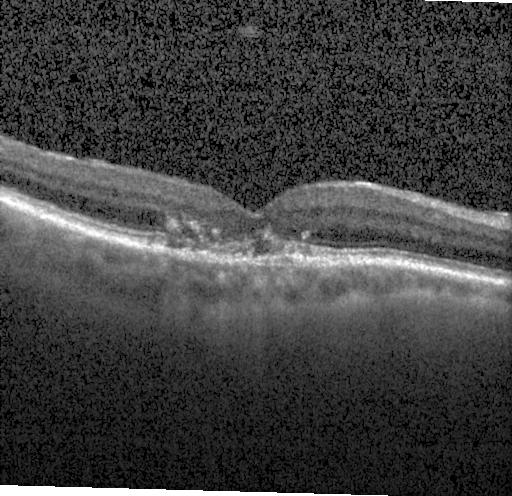
OCT line scan · instrument: Heidelberg Spectralis
OCT finding: a choroidal neovascular membrane.